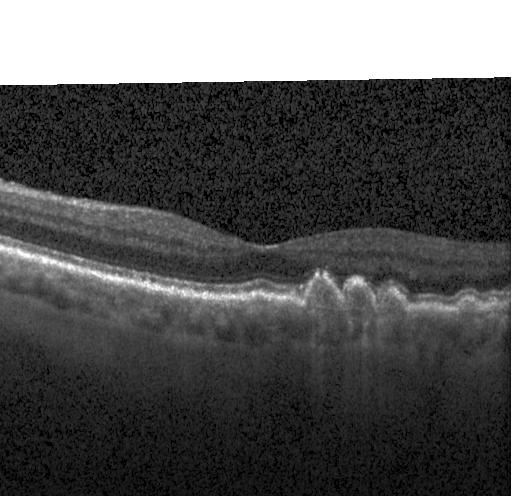
Through the macula. Acquired on a Heidelberg Spectralis. Retinal OCT B-scan. The scan shows multiple drusen.